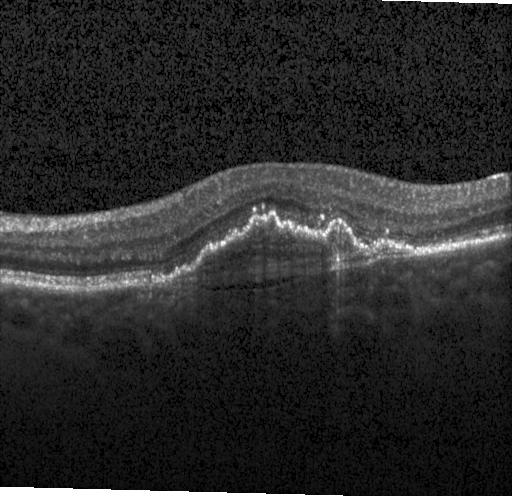

A choroidal neovascular membrane.